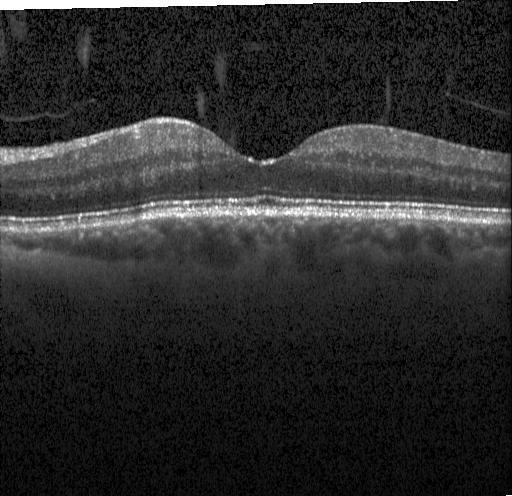

Retinal OCT B-scan, horizontal scan through the fovea.
This B-scan demonstrates no choroidal neovascularization, no diabetic macular edema, and no drusen.